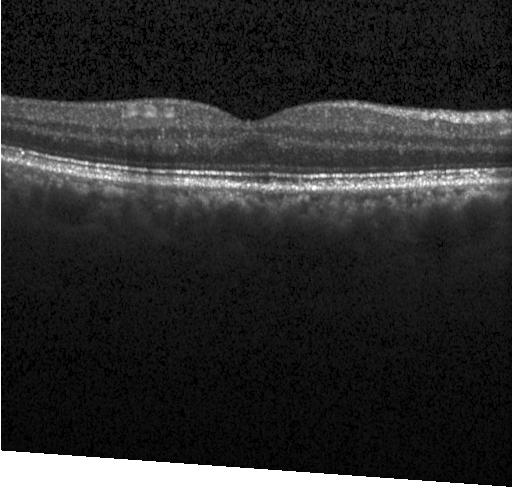
OCT B-scan. Macular scan.
Macular OCT: no choroidal neovascularization, diabetic macular edema, or drusen.